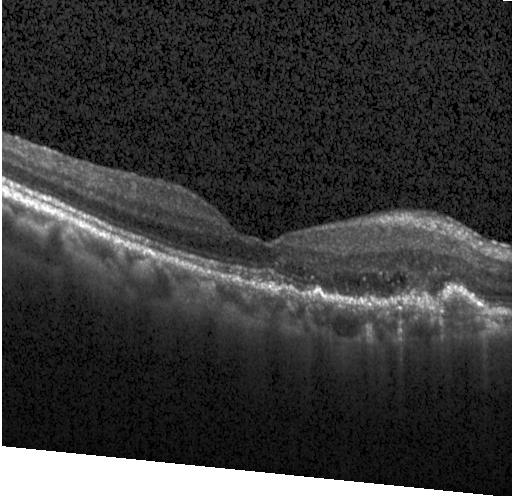
OCT B-scan.
OCT finding: a choroidal neovascular membrane.